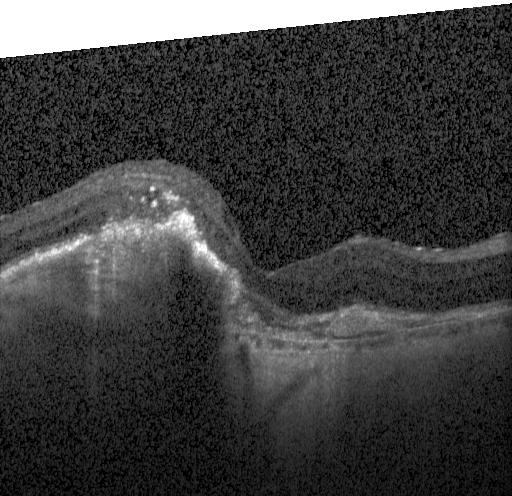

OCT B-scan showing CNV.